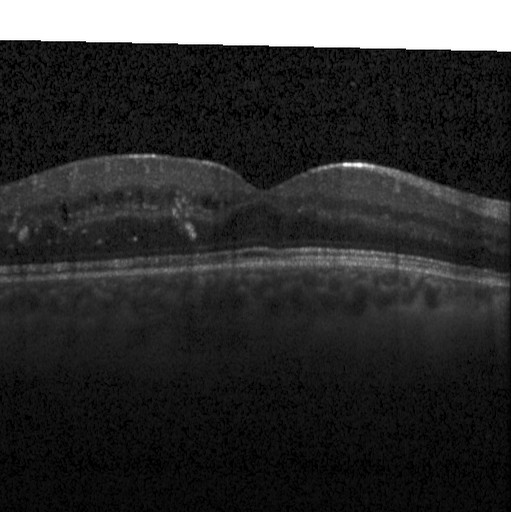 Optical coherence tomography B-scan · spectral-domain OCT
Finding: diabetic macular edema.